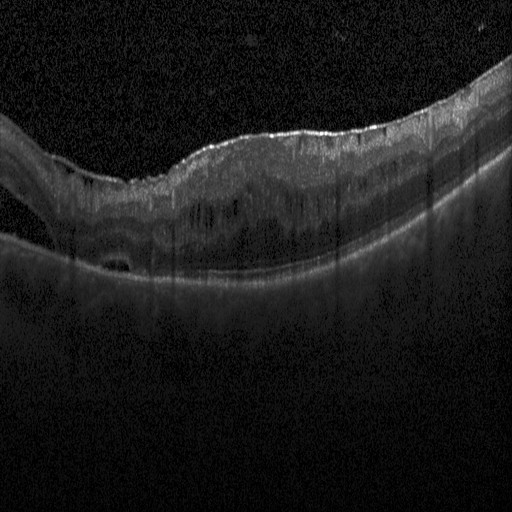
Impression: diabetic macular edema (DME).